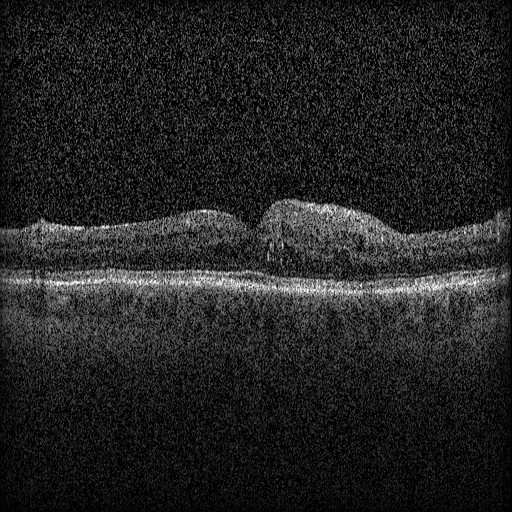 Macular OCT demonstrating diabetic macular edema (DME).